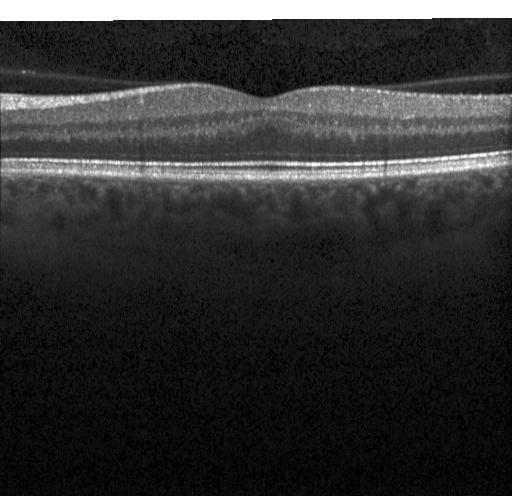 Optical coherence tomography scan · SD-OCT · Heidelberg Spectralis OCT system.
Dx: neither choroidal neovascularization, diabetic macular edema, nor drusen.